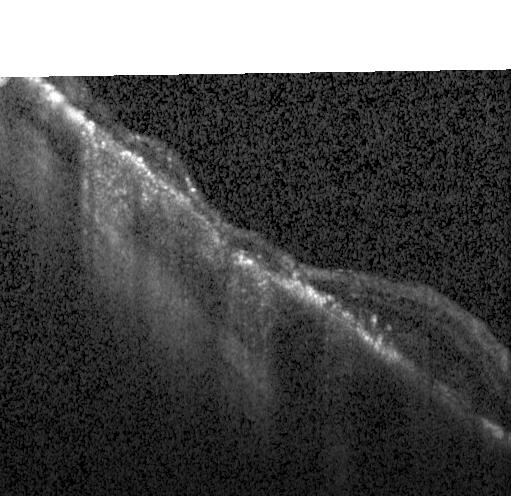
OCT line scan · spectral-domain OCT.
Impression: choroidal neovascularization.